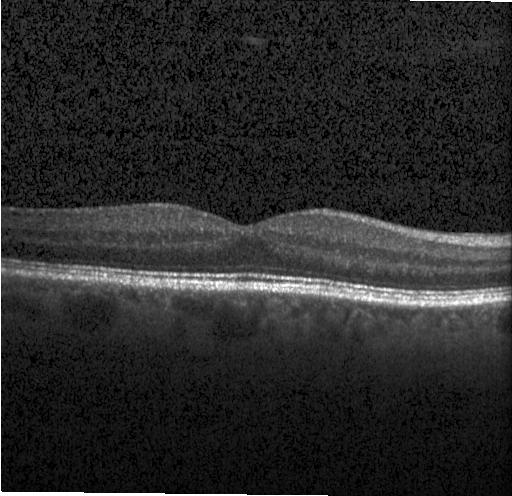 Assessment: neither choroidal neovascularization, diabetic macular edema, nor drusen.